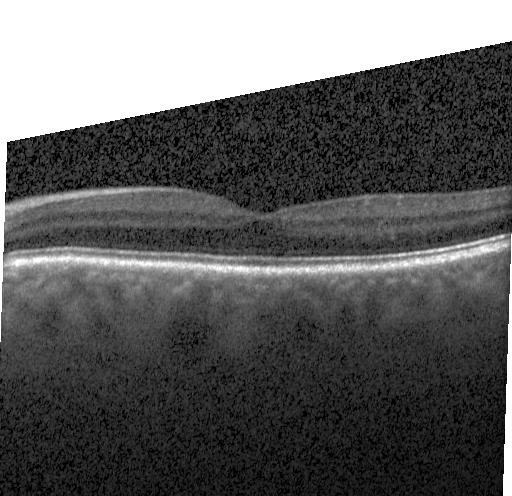
Optical coherence tomography scan. Instrument: Heidelberg Spectralis
Neither CNV, DME, nor drusen.